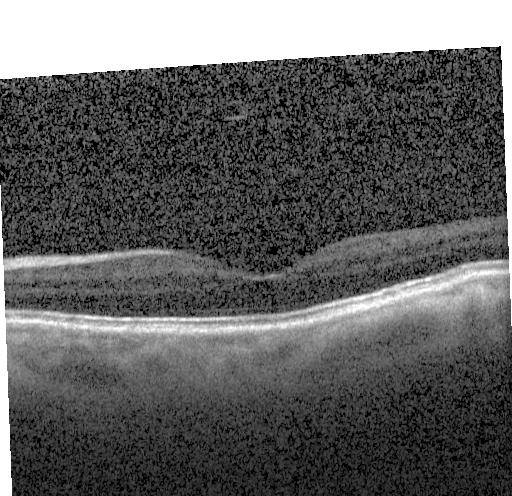 Optical coherence tomography scan, horizontal scan through the fovea, Heidelberg Spectralis OCT system, spectral-domain OCT
Impression: no evidence of CNV, DME, or drusen.